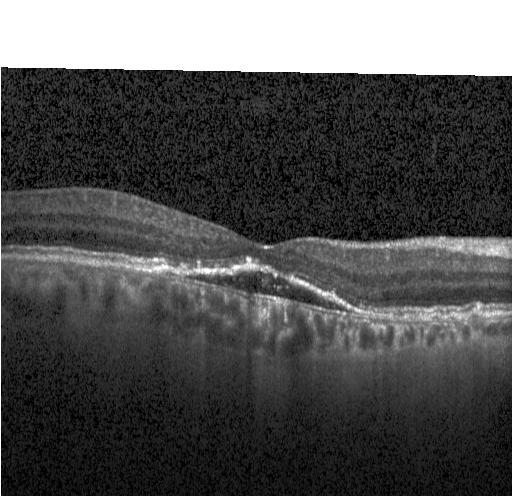

This B-scan demonstrates a choroidal neovascular membrane.